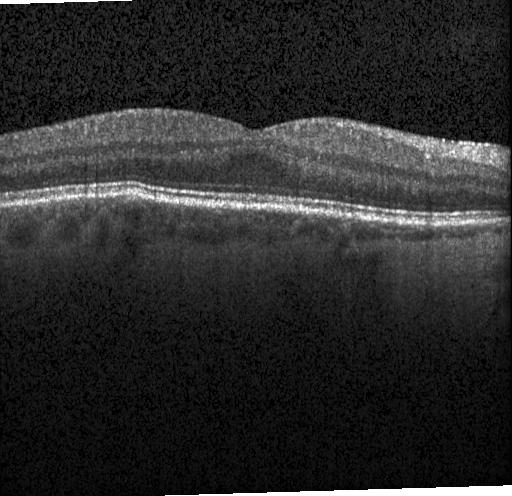 SD-OCT. Retinal OCT B-scan. Through the macula
OCT finding: neither choroidal neovascularization, diabetic macular edema, nor drusen.